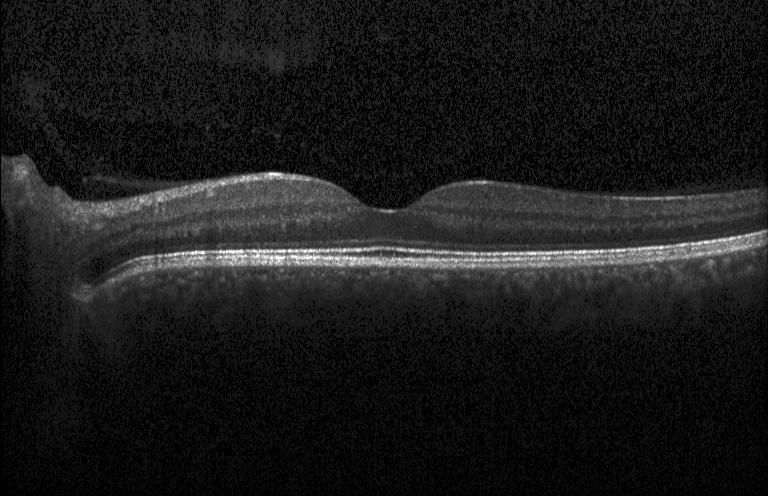

Fovea-centered, optical coherence tomography B-scan, Heidelberg Spectralis OCT system. Assessment: no CNV, no DME, and no drusen.